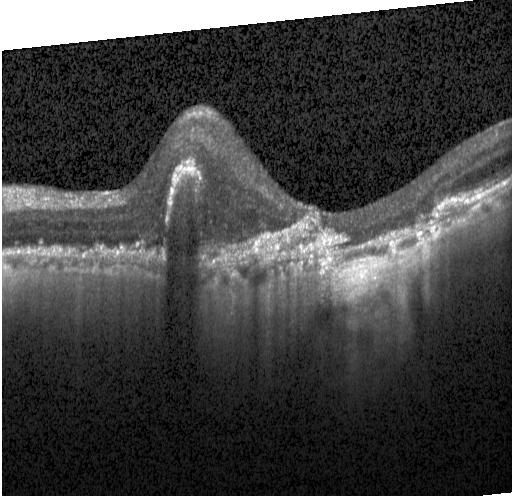 OCT finding: choroidal neovascularization.